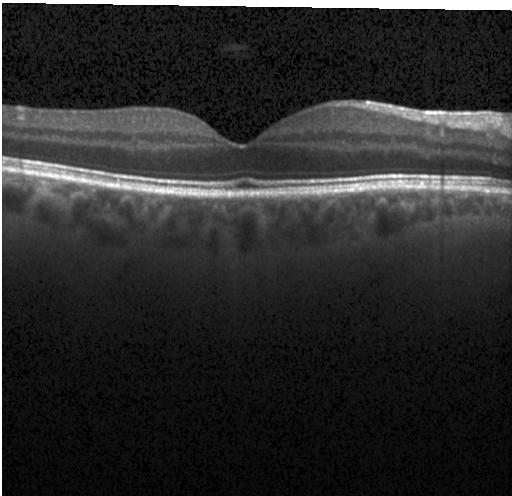 Macular OCT demonstrating neither CNV, DME, nor drusen.